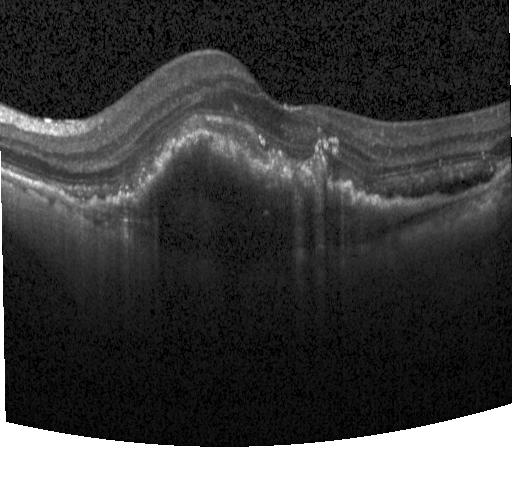
Impression: a choroidal neovascular membrane.